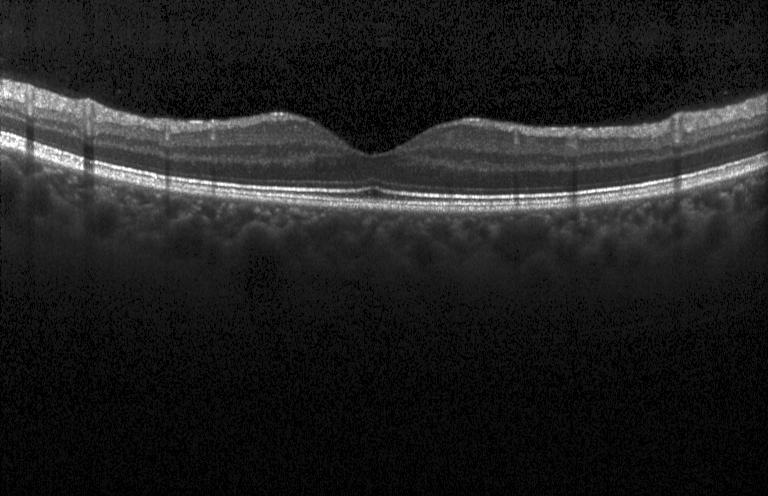 Optical coherence tomography B-scan. Impression: neither choroidal neovascularization, diabetic macular edema, nor drusen.